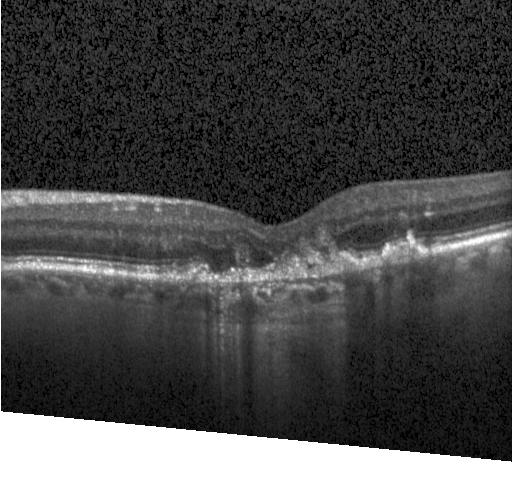 Retinal OCT B-scan · horizontal scan through the fovea · acquired on a Heidelberg Spectralis
This B-scan demonstrates choroidal neovascularization (CNV).